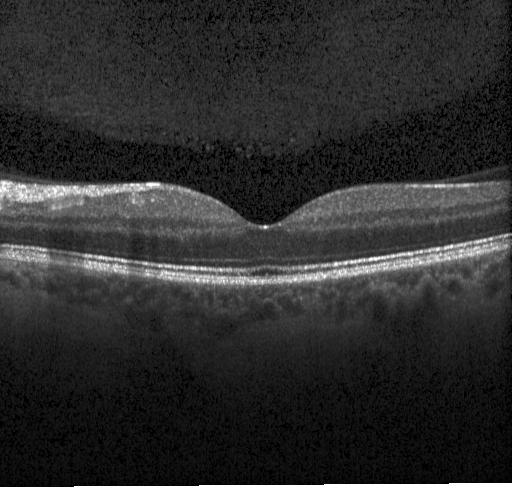 Retinal OCT cross-section, fovea-centered, Heidelberg Spectralis OCT system. Assessment: no CNV, no DME, and no drusen.